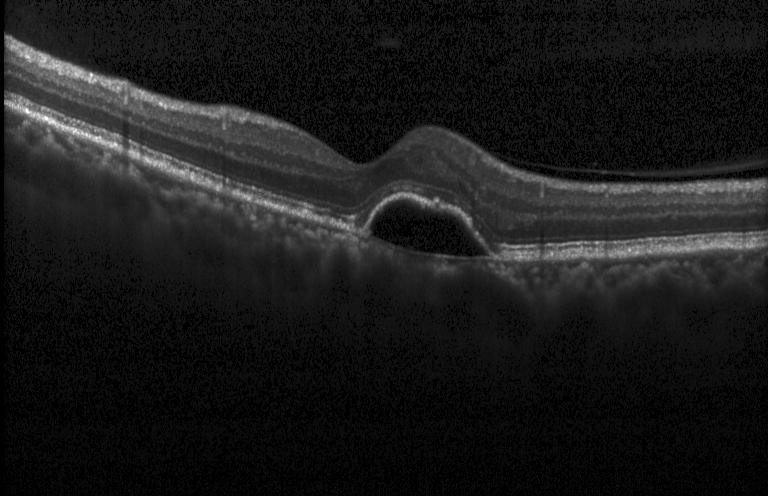 Optical coherence tomography B-scan. Acquired on a Heidelberg Spectralis.
Finding: choroidal neovascularization (CNV).